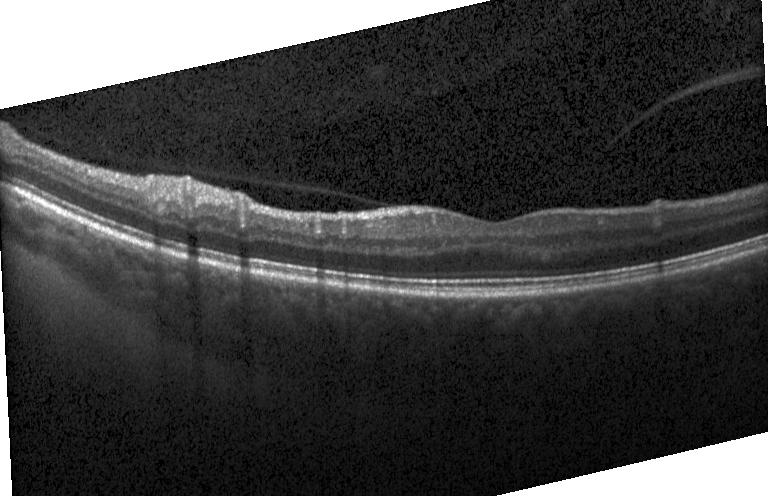 Optical coherence tomography scan
Finding: neither choroidal neovascularization, diabetic macular edema, nor drusen.